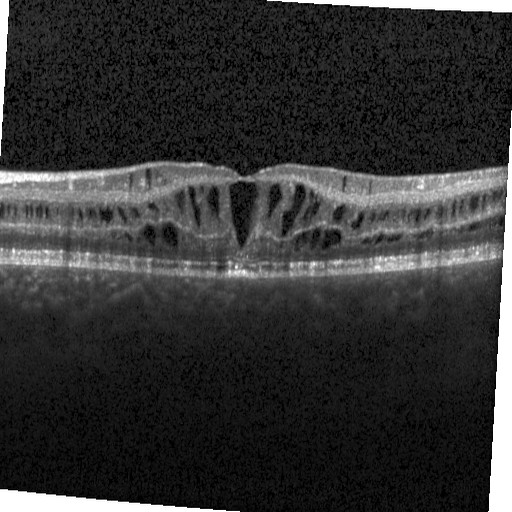 Diagnosis: DME.